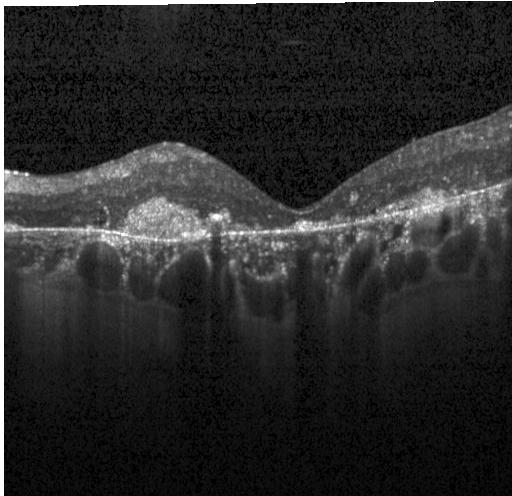

Through the macula; OCT B-scan. Diagnosis: a choroidal neovascular membrane.